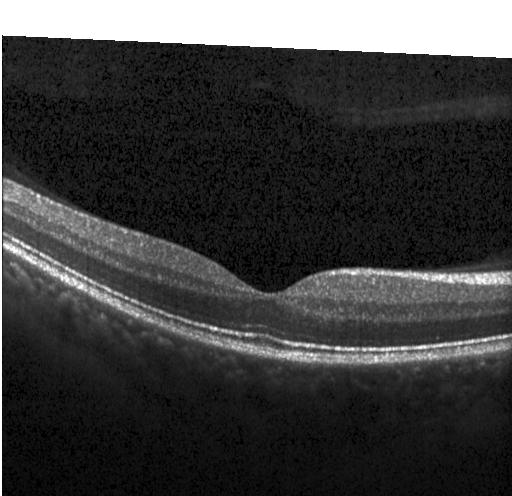
Instrument: Heidelberg Spectralis; retinal OCT B-scan
The scan shows no choroidal neovascularization, no diabetic macular edema, and no drusen.